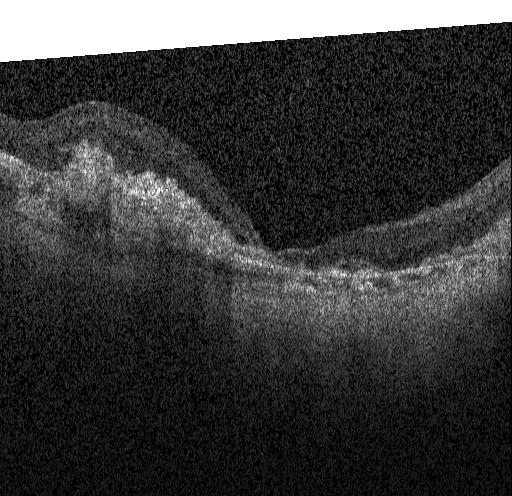

Heidelberg Spectralis, through the macula, OCT B-scan.
A choroidal neovascular membrane.